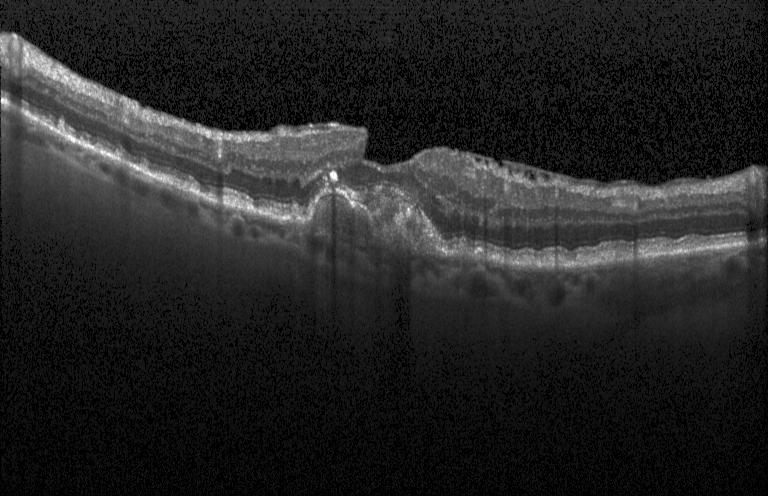 Macular scan. OCT line scan. Acquired on a Heidelberg Spectralis. Spectral-domain optical coherence tomography.
Impression: choroidal neovascularization (CNV).